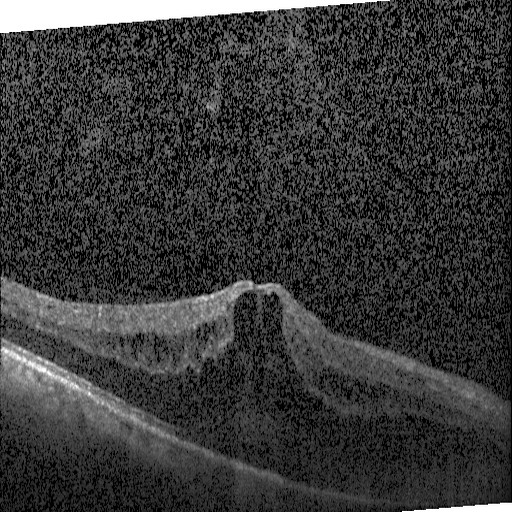
Impression: diabetic macular edema.